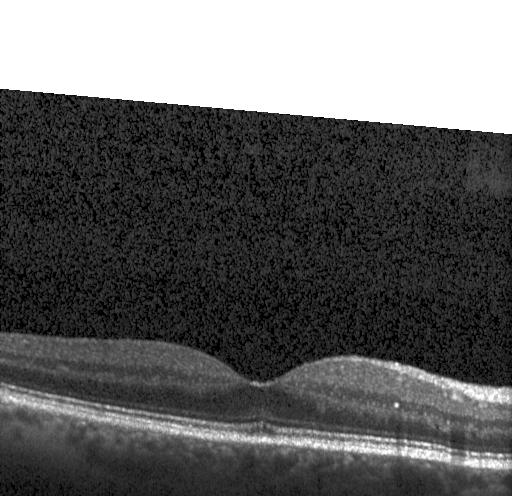

OCT line scan.
Impression: no choroidal neovascularization, diabetic macular edema, or drusen.